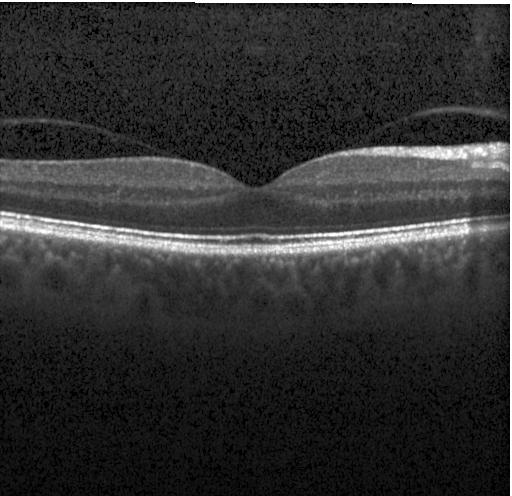 OCT finding: no evidence of CNV, DME, or drusen.